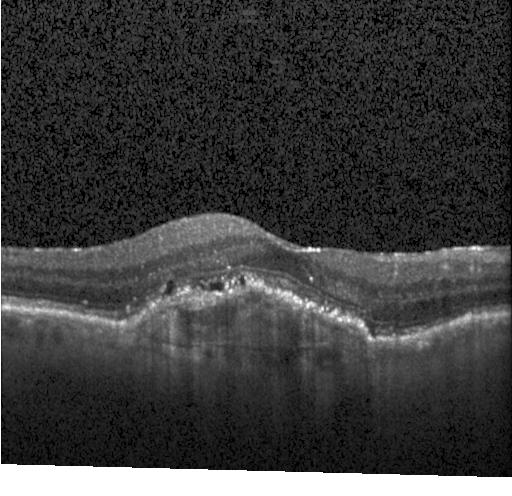 Dx: choroidal neovascularization.